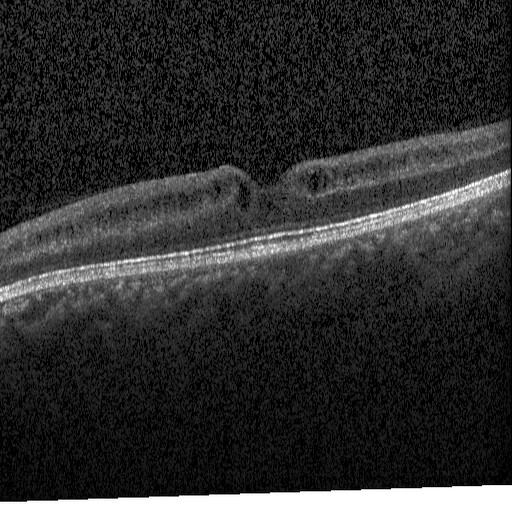
Instrument: Heidelberg Spectralis, optical coherence tomography scan, through the macula. Finding: diabetic macular edema (DME).